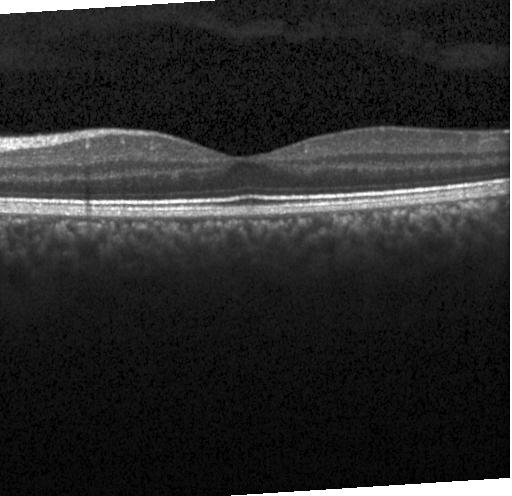
OCT line scan; instrument: Heidelberg Spectralis
Diagnosis: no CNV, no DME, and no drusen.